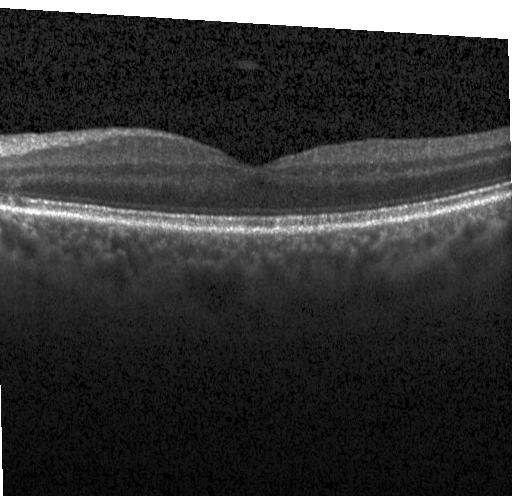

SD-OCT; retinal OCT B-scan
No choroidal neovascularization, diabetic macular edema, or drusen.